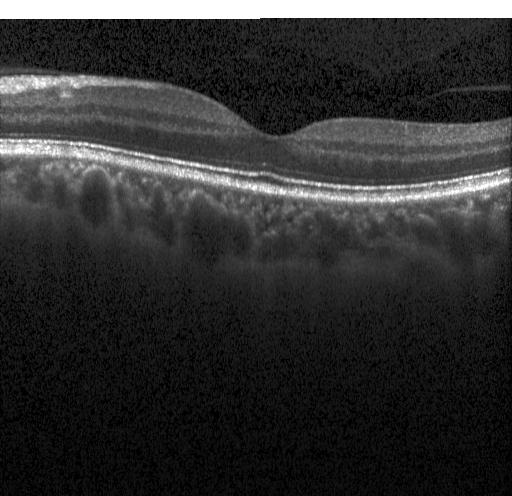 Optical coherence tomography B-scan; through the macula; spectral-domain optical coherence tomography
Diagnosis: no evidence of CNV, DME, or drusen.